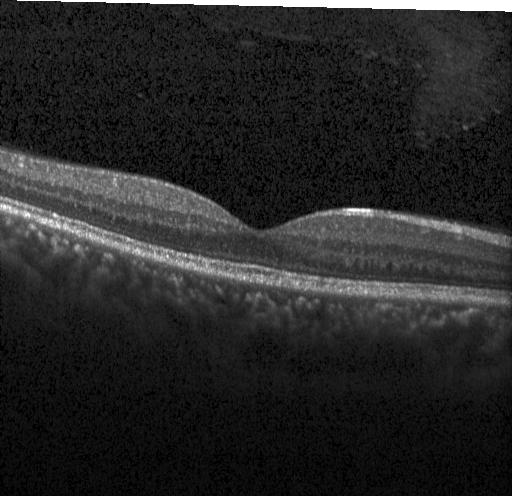
OCT B-scan, acquired on a Heidelberg Spectralis, horizontal scan through the fovea
Macular OCT: no CNV, no DME, and no drusen.